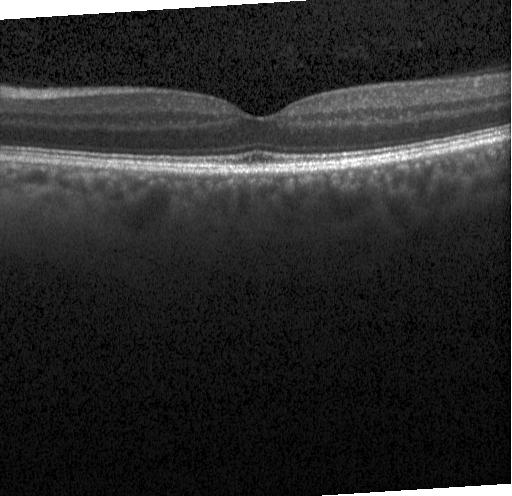 Spectral-domain optical coherence tomography · optical coherence tomography scan
Impression: no CNV, DME, or drusen.